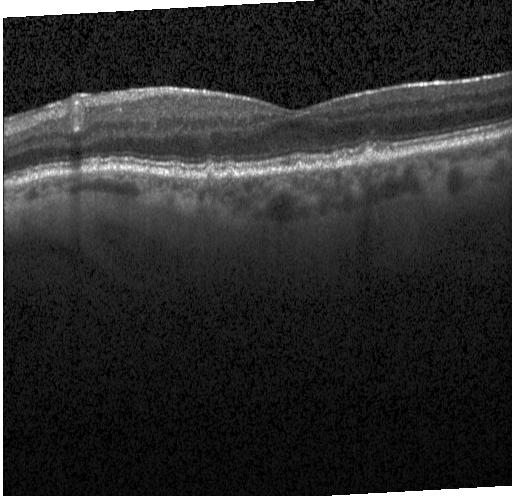
Spectral-domain OCT; retinal OCT B-scan.
Sub-RPE drusenoid deposits.